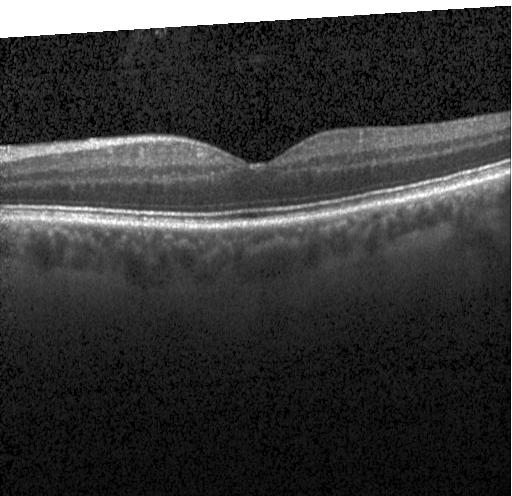

Dx: no choroidal neovascularization, no diabetic macular edema, and no drusen.